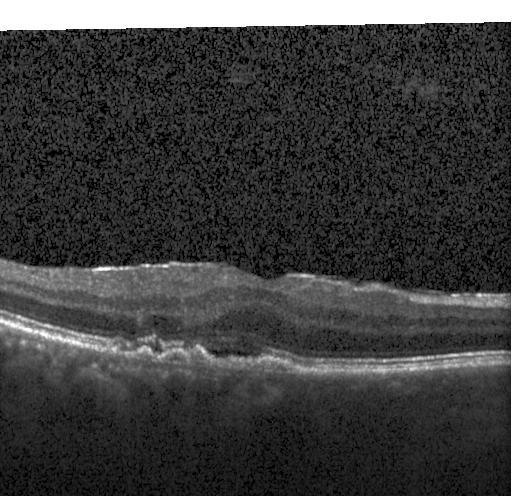
OCT B-scan showing a choroidal neovascular membrane.